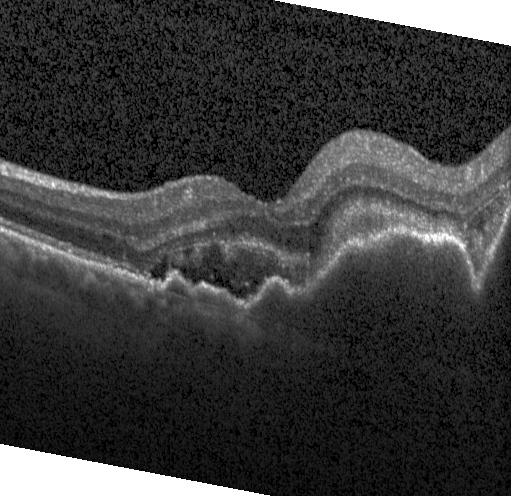
OCT line scan; spectral-domain optical coherence tomography — The scan shows choroidal neovascularization (CNV).